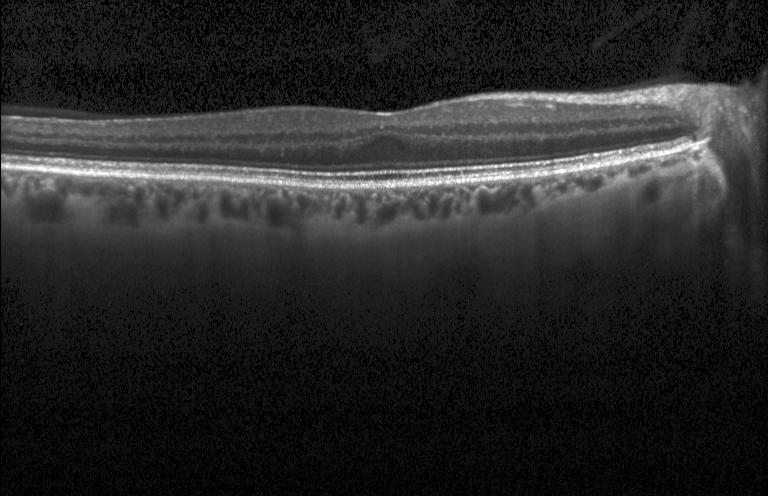
SD-OCT; optical coherence tomography scan; instrument: Heidelberg Spectralis.
Diagnosis: no evidence of CNV, DME, or drusen.